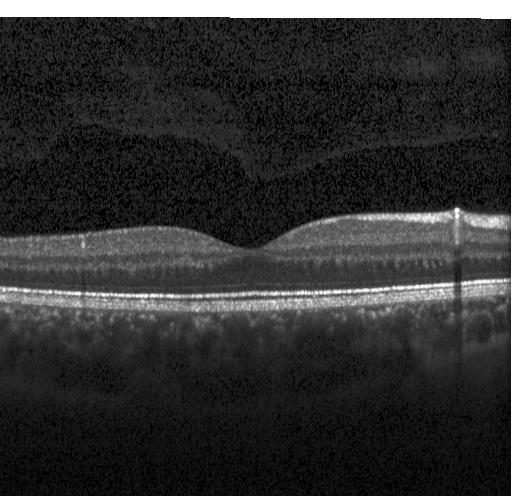

Impression: no evidence of choroidal neovascularization, diabetic macular edema, or drusen.